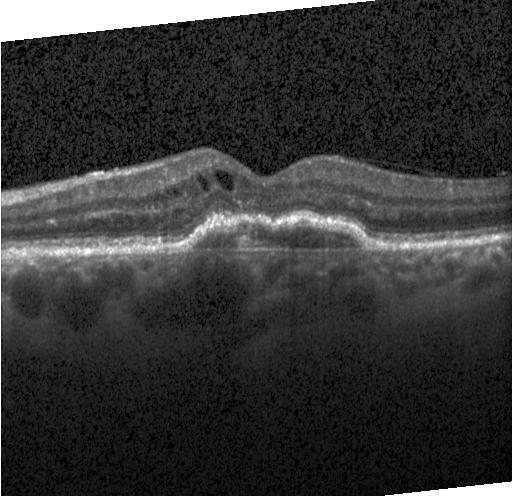 Retinal OCT B-scan, fovea-centered, spectral-domain OCT, Heidelberg Spectralis OCT system — Impression: a choroidal neovascular membrane.